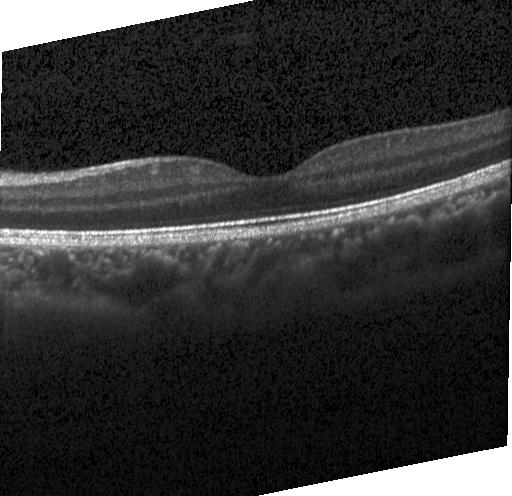 Macular OCT: neither choroidal neovascularization, diabetic macular edema, nor drusen.